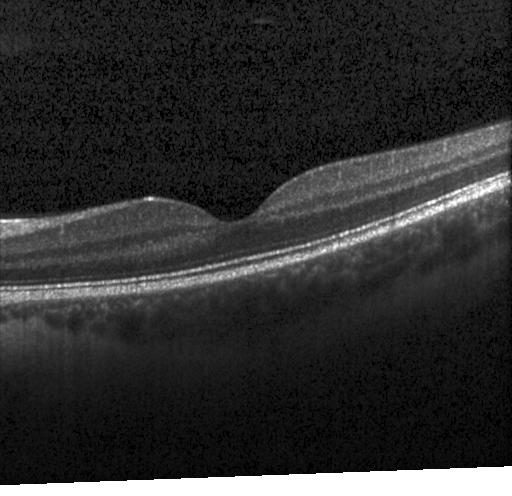 Finding: no choroidal neovascularization, no diabetic macular edema, and no drusen.